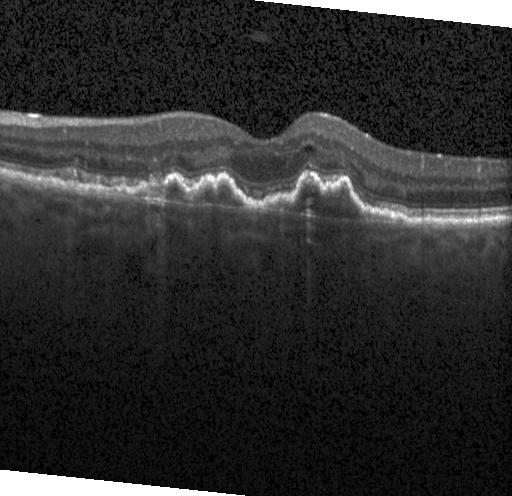 Diagnosis: choroidal neovascularization (CNV).